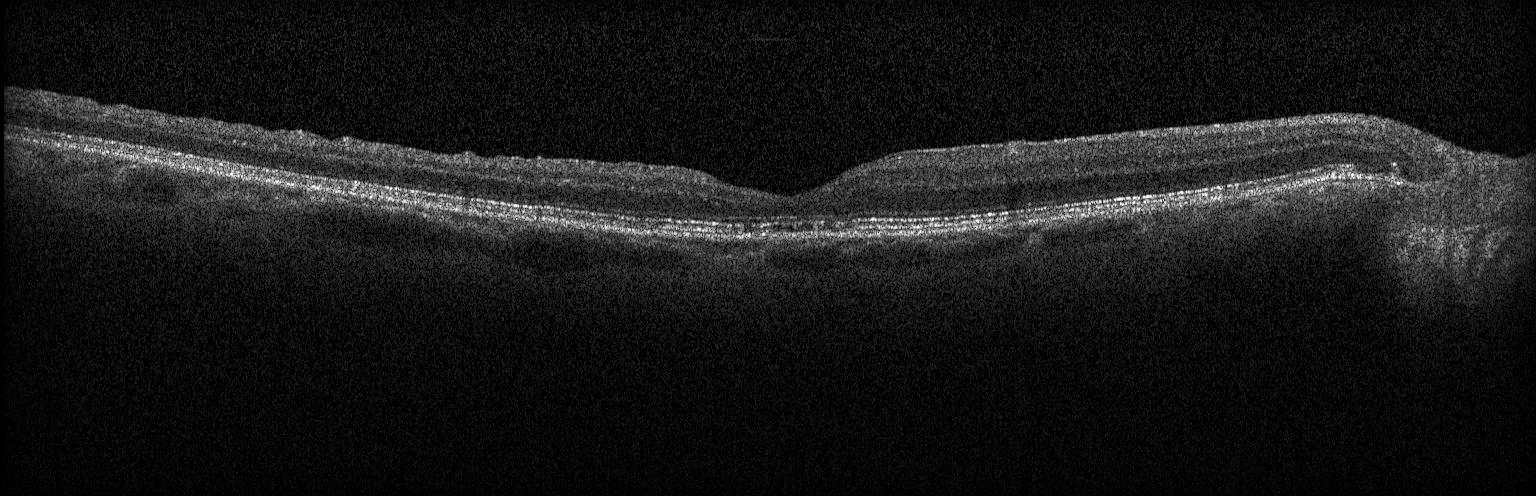

Spectral-domain OCT; OCT B-scan; Heidelberg Spectralis
Diagnosis: no CNV, no DME, and no drusen.